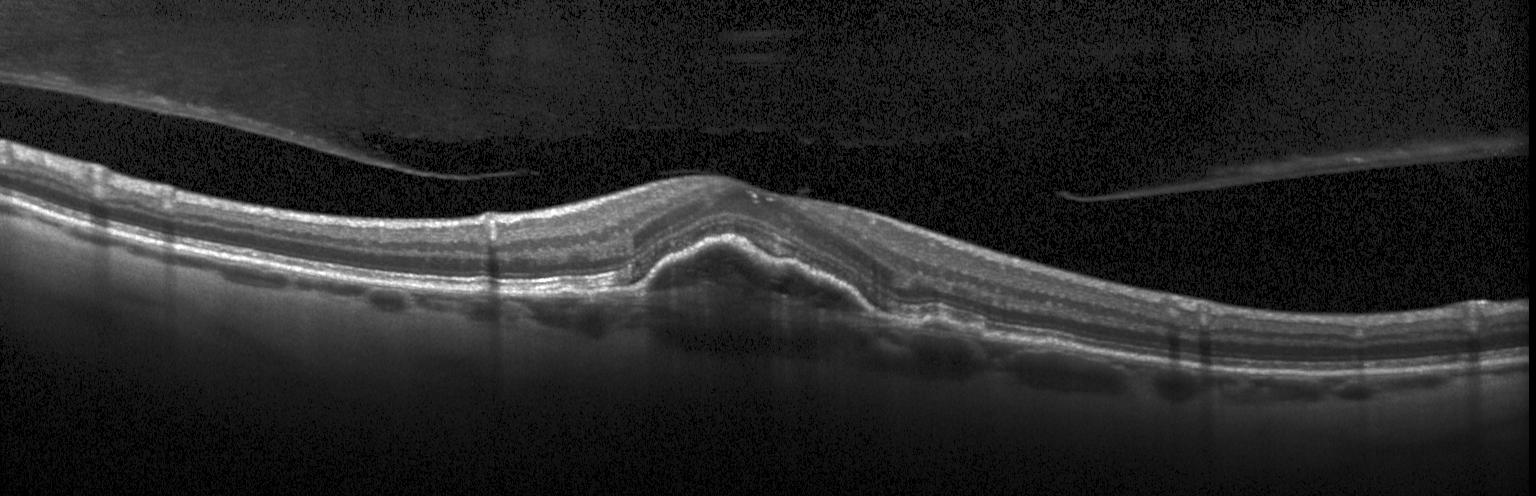

Spectral-domain OCT B-scan: a choroidal neovascular membrane.